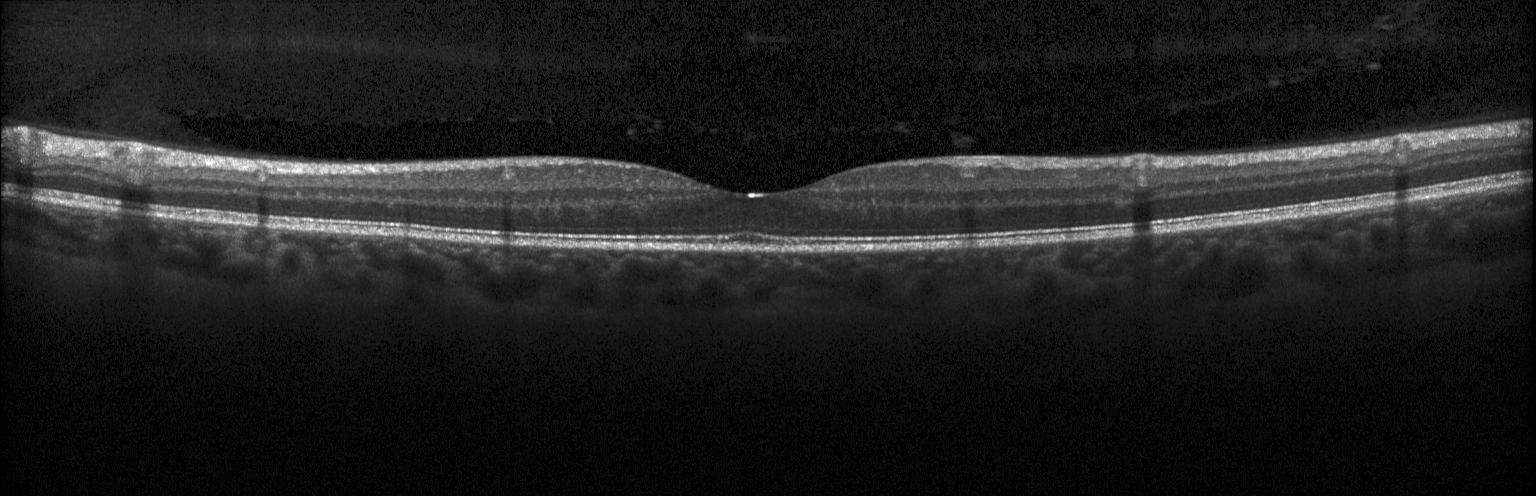 Assessment: no choroidal neovascularization, diabetic macular edema, or drusen.